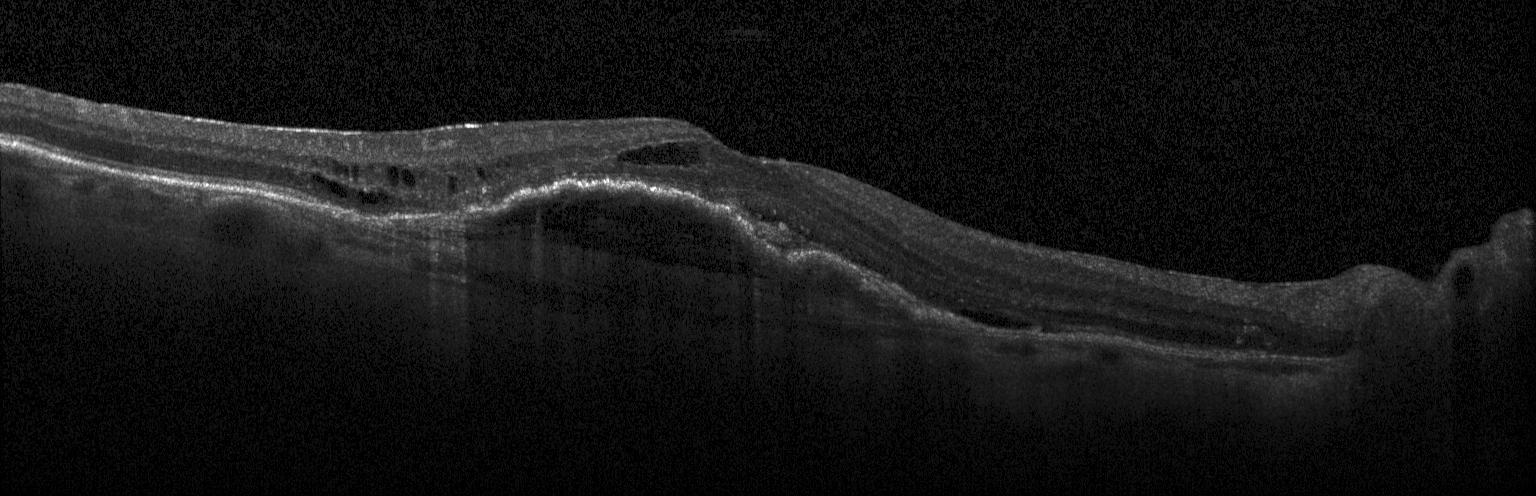
Diagnosis: choroidal neovascularization.